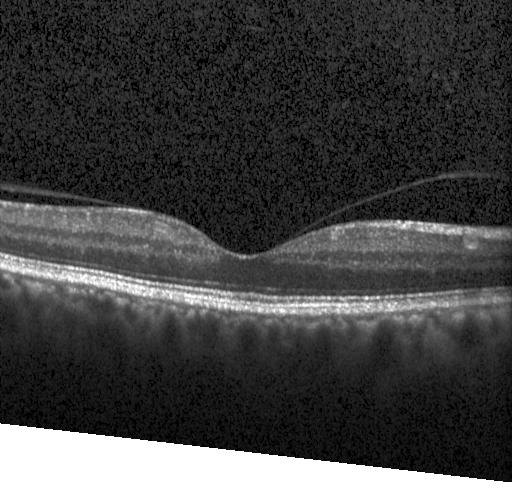 Instrument: Heidelberg Spectralis, OCT B-scan — Impression: no choroidal neovascularization, diabetic macular edema, or drusen.